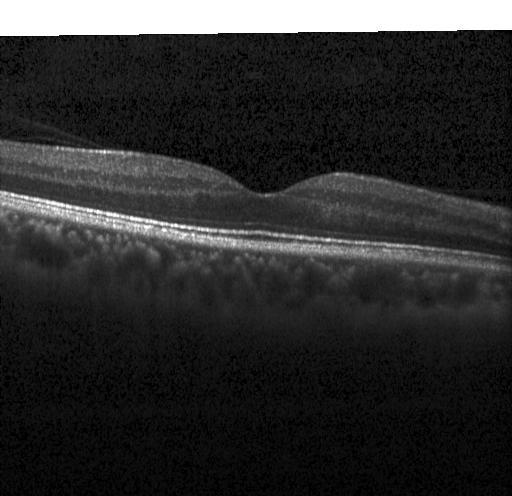
OCT B-scan. Through the macula — OCT finding: neither CNV, DME, nor drusen.